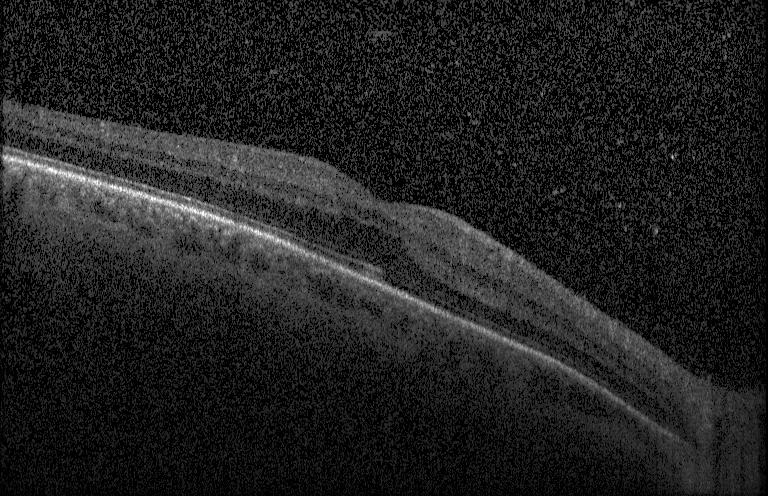
Spectral-domain OCT, retinal OCT B-scan, fovea-centered, acquired on a Heidelberg Spectralis. No CNV, no DME, and no drusen.